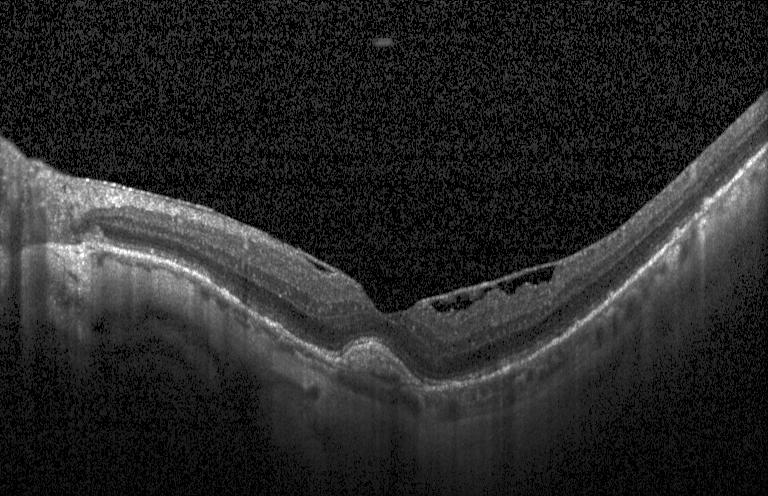
Fovea-centered. SD-OCT. Retinal OCT B-scan. Instrument: Heidelberg Spectralis
Choroidal neovascularization.